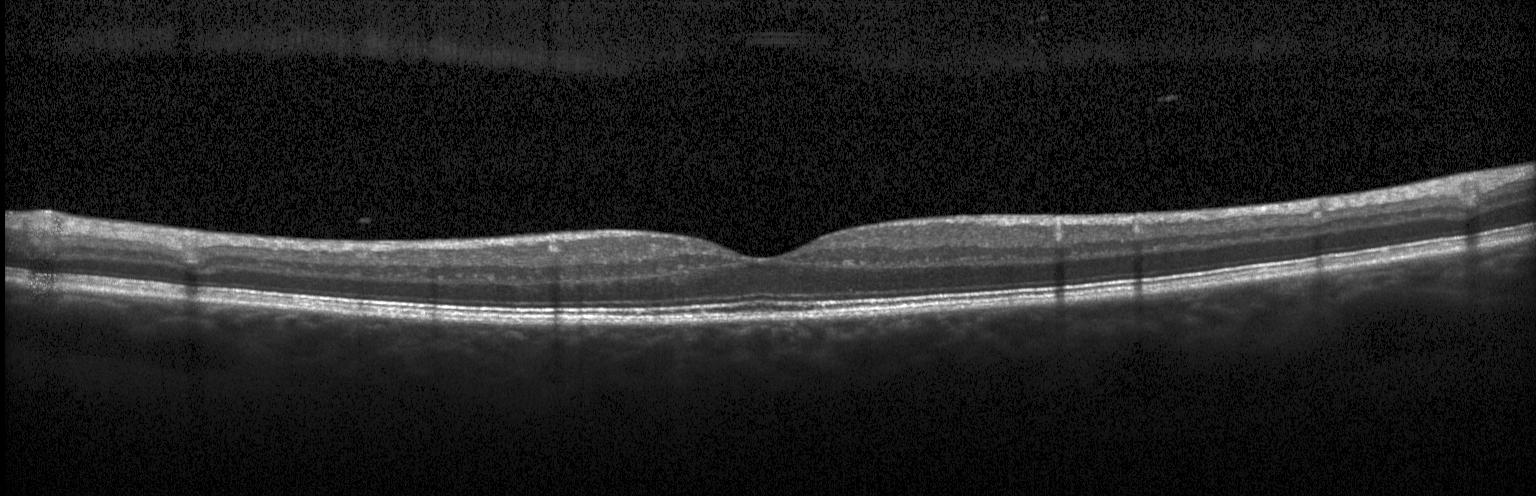

Macular OCT demonstrating no CNV, no DME, and no drusen.